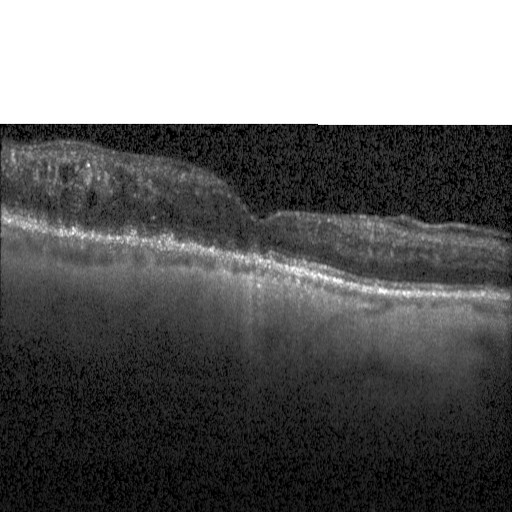 Heidelberg Spectralis; optical coherence tomography scan. Finding: diabetic macular edema.